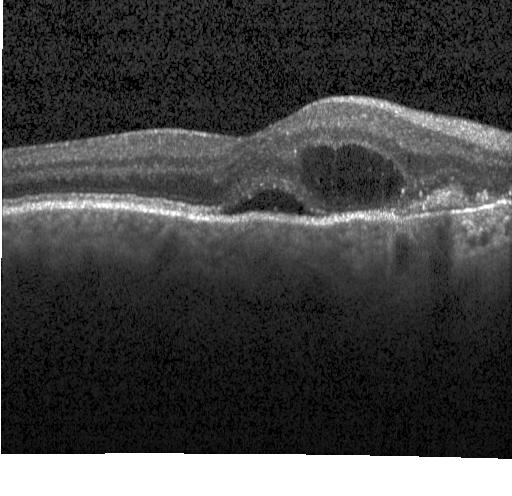

OCT finding: choroidal neovascularization.